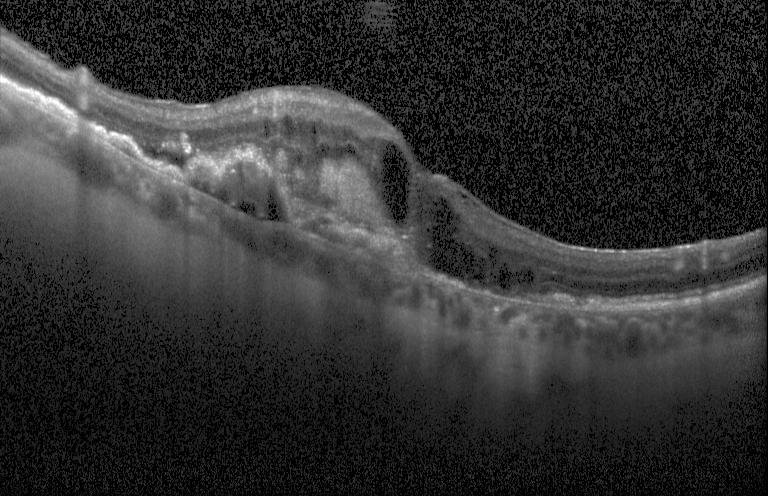
Through the macula, optical coherence tomography B-scan. Assessment: a choroidal neovascular membrane.